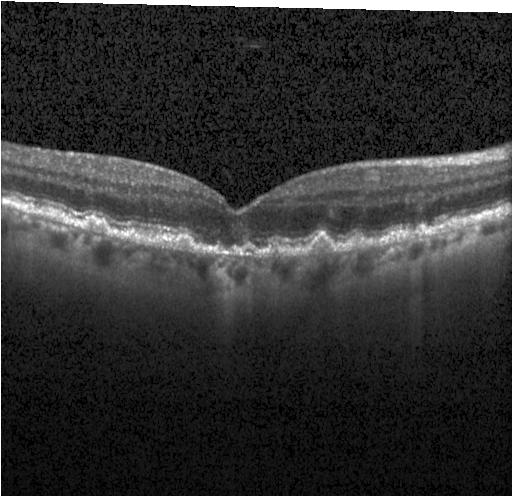 Spectral-domain OCT. Retinal OCT cross-section — Dx: sub-RPE drusenoid deposits.